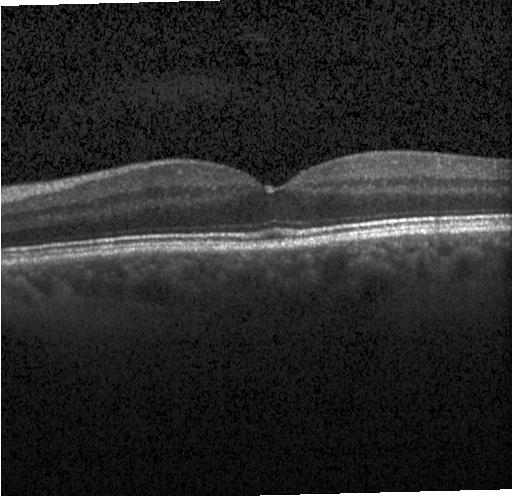

Spectral-domain optical coherence tomography; retinal OCT cross-section; centered on the fovea.
The scan shows no evidence of choroidal neovascularization, diabetic macular edema, or drusen.